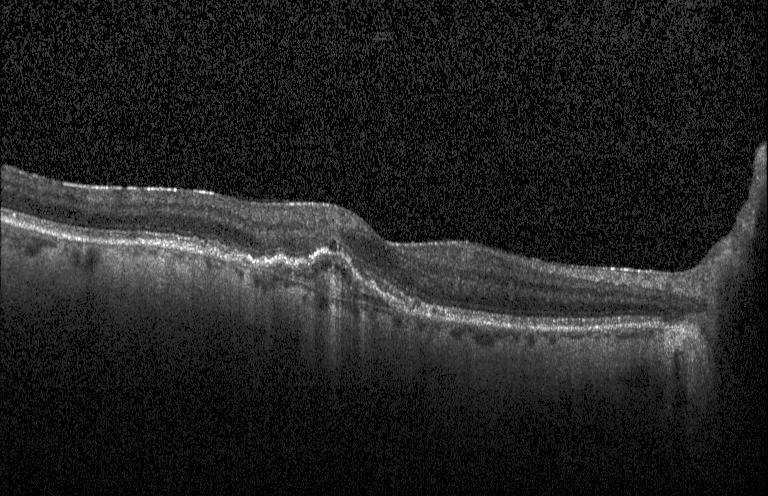
Optical coherence tomography B-scan
OCT finding: a choroidal neovascular membrane.